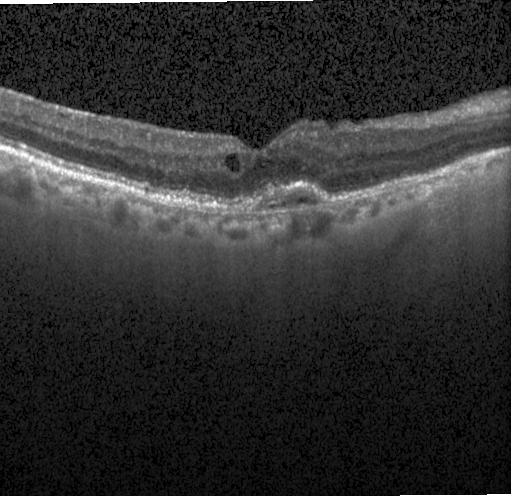
Finding: choroidal neovascularization.